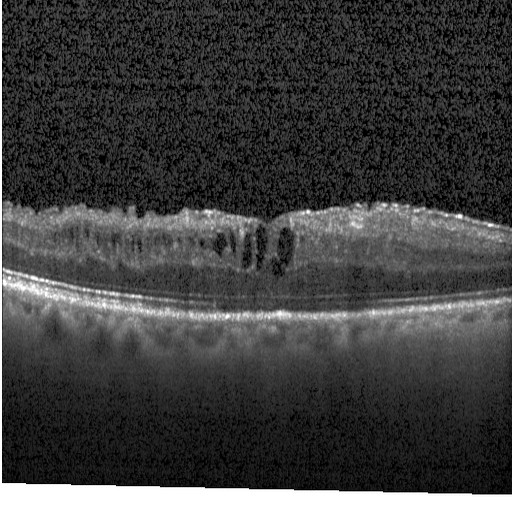 Fovea-centered · instrument: Heidelberg Spectralis · spectral-domain OCT · retinal OCT cross-section — Impression: DME.